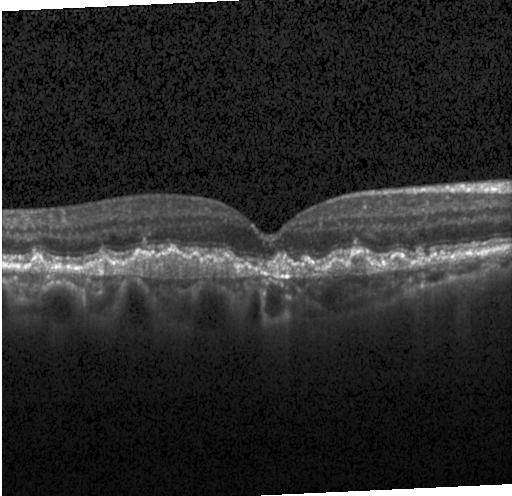

Diagnosis: a choroidal neovascular membrane.